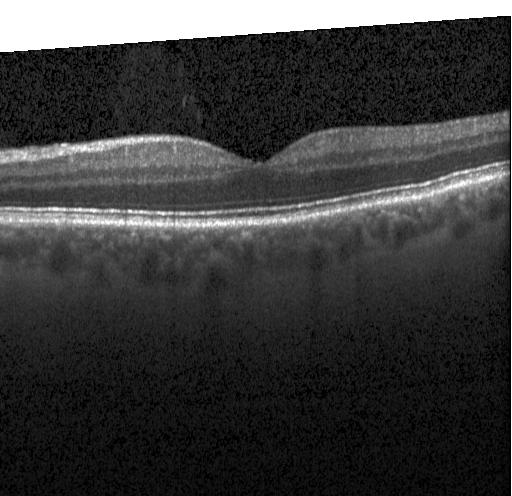

Spectral-domain OCT; retinal OCT cross-section.
Diagnosis: neither choroidal neovascularization, diabetic macular edema, nor drusen.